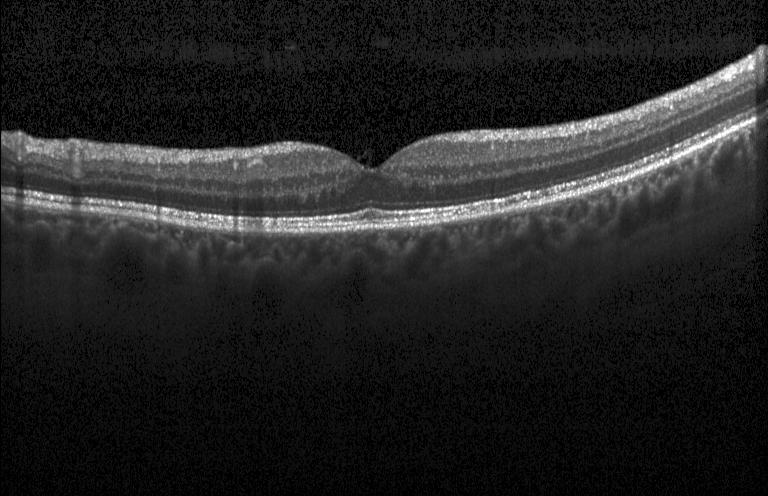 Spectral-domain OCT; OCT B-scan
Finding: no evidence of CNV, DME, or drusen.